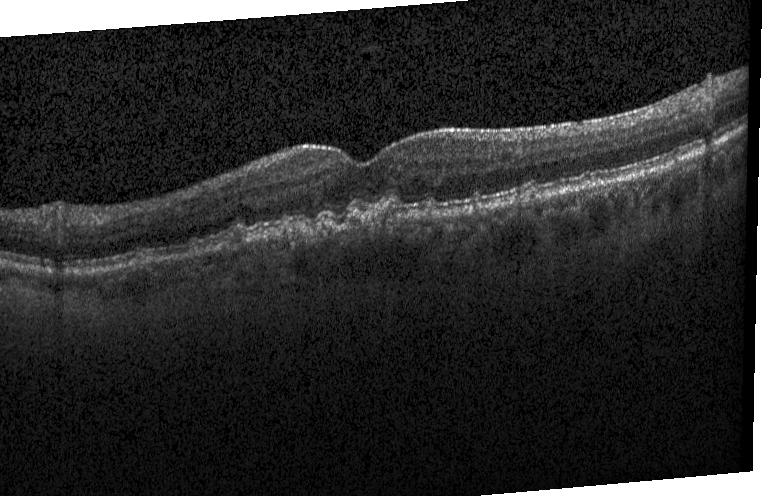

Retinal OCT cross-section. Multiple drusen.